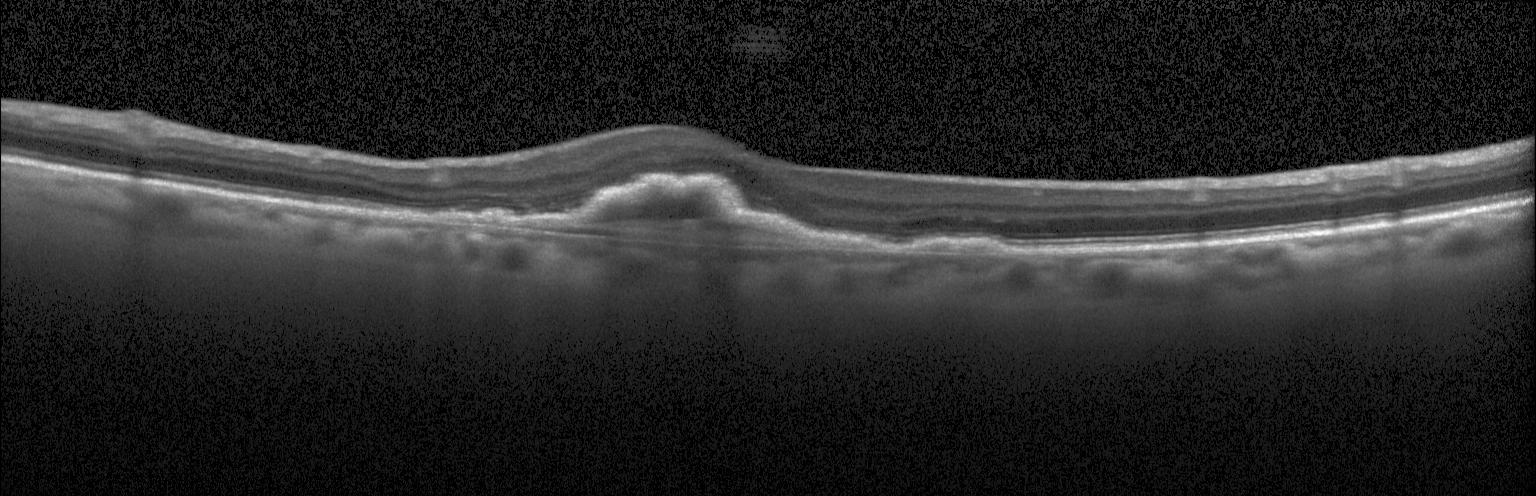 Spectral-domain OCT. OCT line scan — Assessment: choroidal neovascularization.